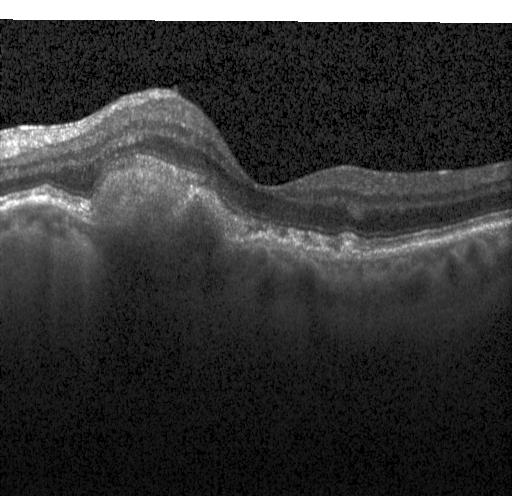
Optical coherence tomography scan. This B-scan demonstrates CNV.